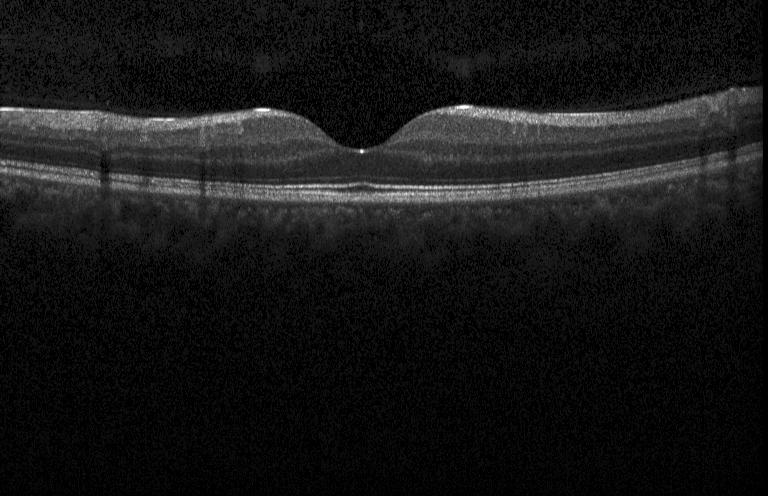

Optical coherence tomography B-scan. Diagnosis: neither CNV, DME, nor drusen.